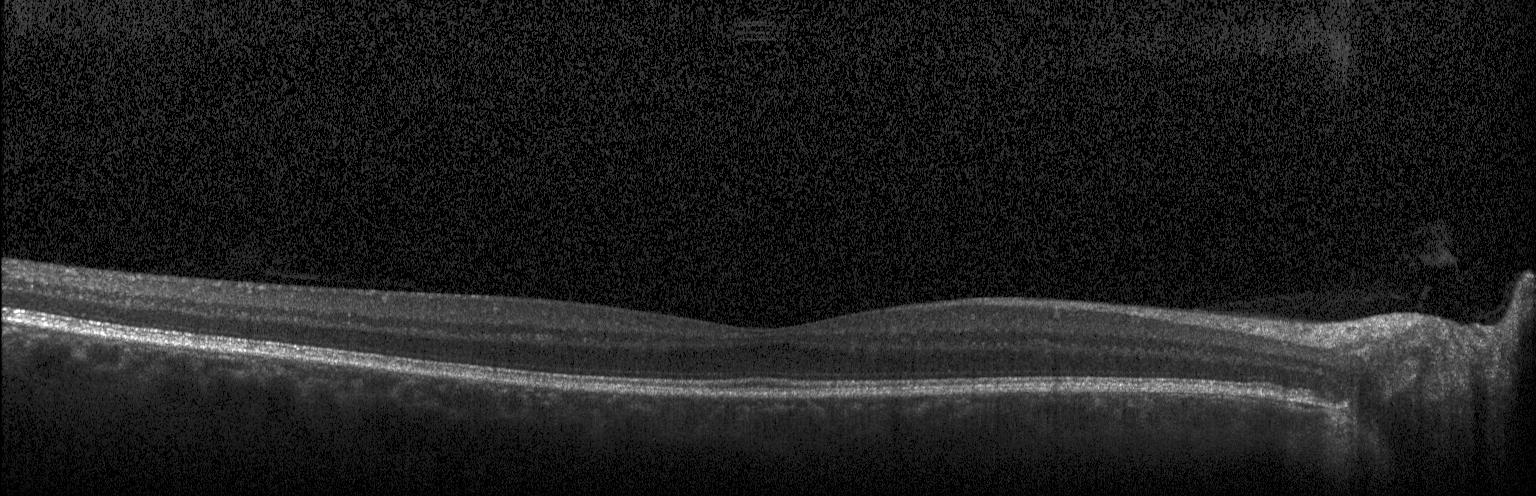

OCT finding: neither CNV, DME, nor drusen.